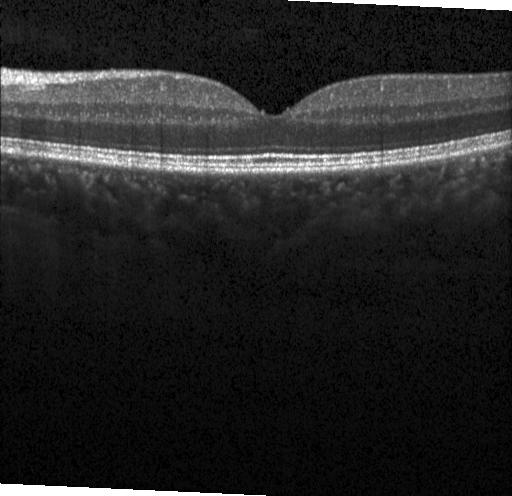

Horizontal scan through the fovea. Retinal OCT B-scan. Acquired on a Heidelberg Spectralis. Spectral-domain optical coherence tomography — Impression: no choroidal neovascularization, diabetic macular edema, or drusen.